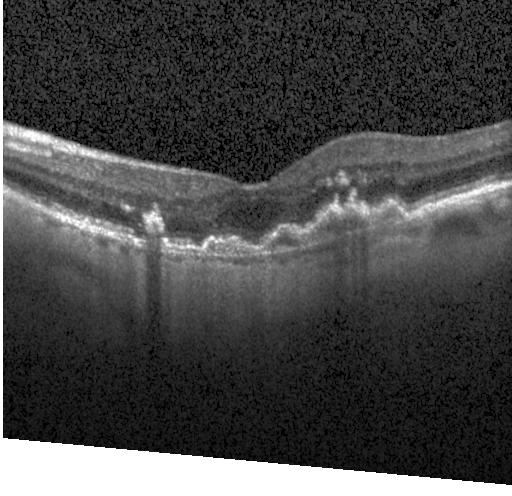
Impression: choroidal neovascularization.